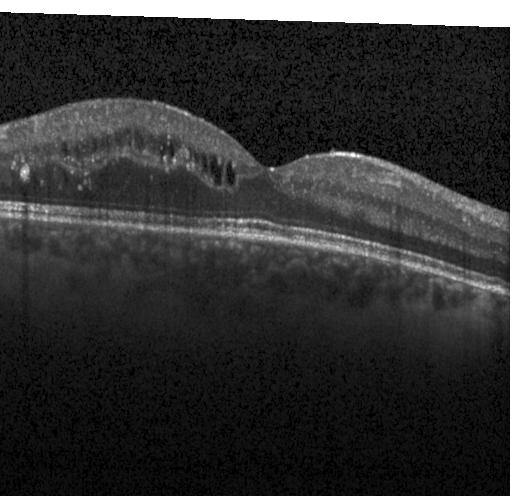
OCT line scan, centered on the fovea, acquired on a Heidelberg Spectralis — This B-scan demonstrates DME.